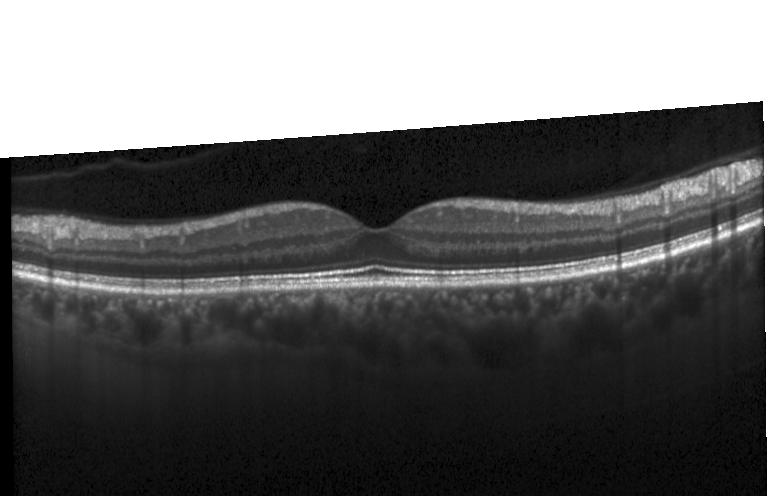
Instrument: Heidelberg Spectralis, optical coherence tomography scan. The scan shows no evidence of CNV, DME, or drusen.